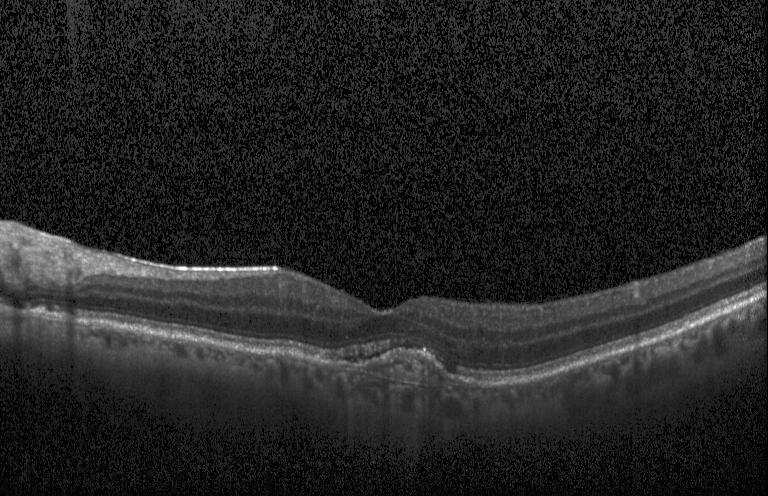
OCT B-scan, spectral-domain optical coherence tomography — Diagnosis: CNV.